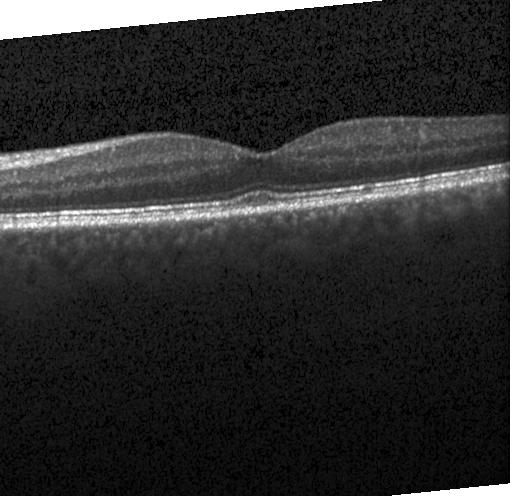 Impression: no choroidal neovascularization, diabetic macular edema, or drusen.